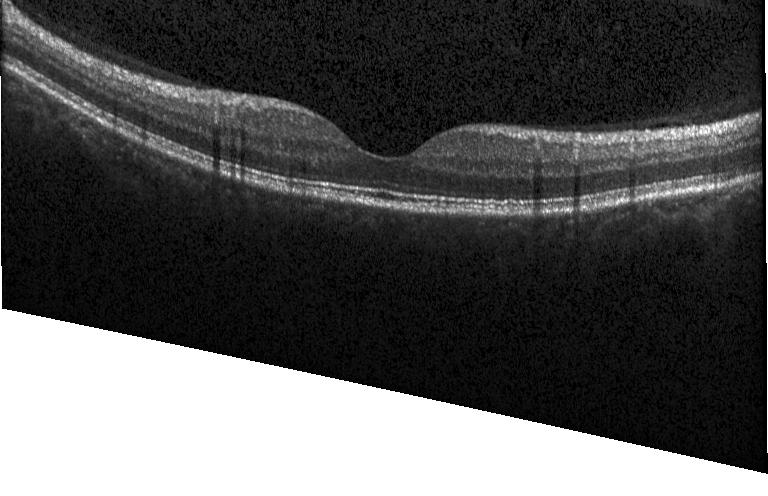
Assessment: no evidence of choroidal neovascularization, diabetic macular edema, or drusen.